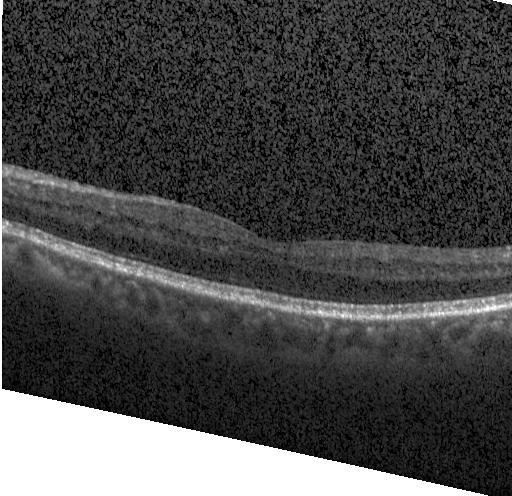
Retinal OCT cross-section.
OCT finding: no CNV, no DME, and no drusen.